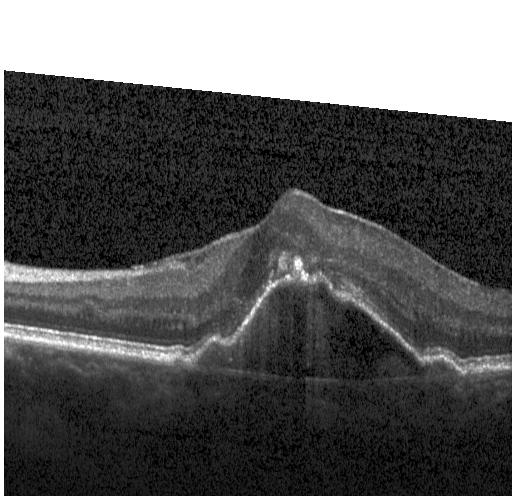
Heidelberg Spectralis OCT system, optical coherence tomography scan, SD-OCT. Impression: a choroidal neovascular membrane.